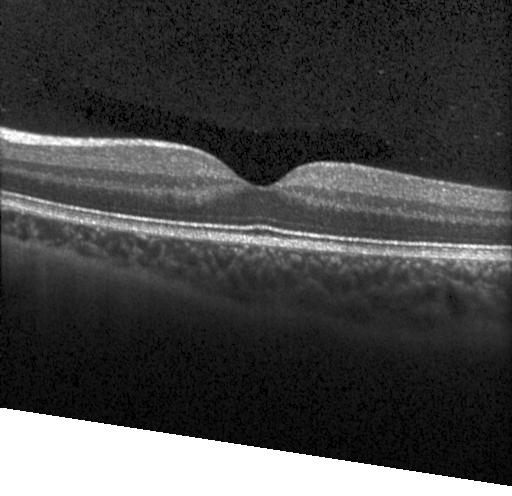

Retinal OCT cross-section showing no CNV, no DME, and no drusen.